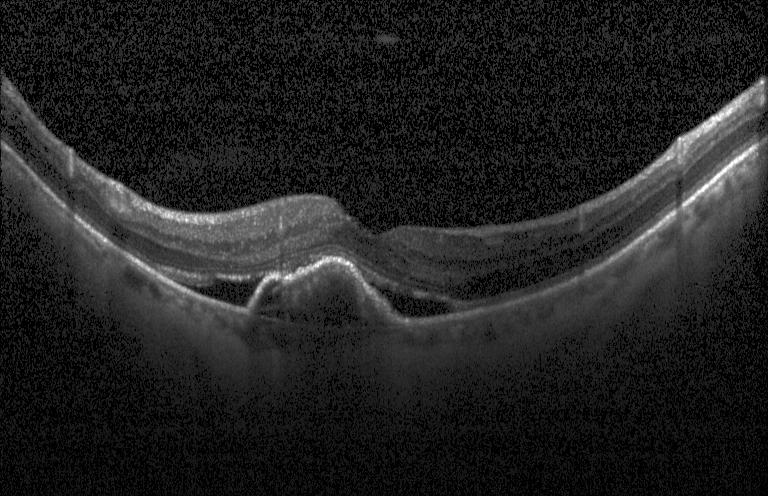
Diagnosis: choroidal neovascularization.